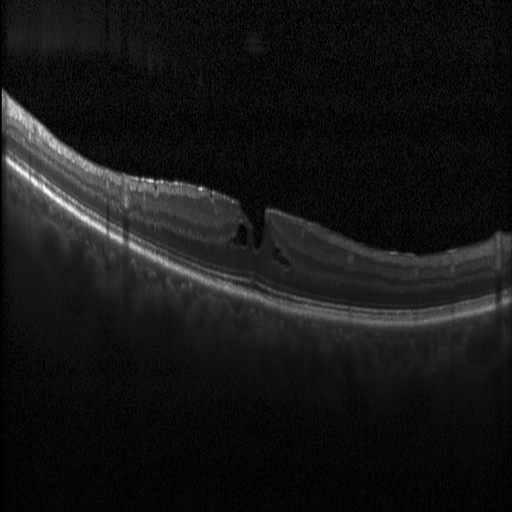
OCT finding: diabetic macular edema (DME).